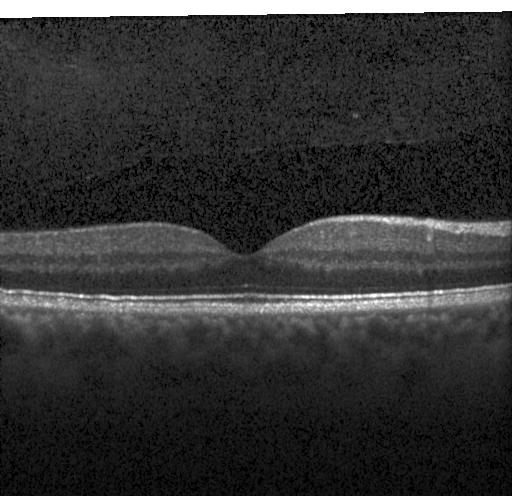 Retinal OCT B-scan.
This B-scan demonstrates neither CNV, DME, nor drusen.